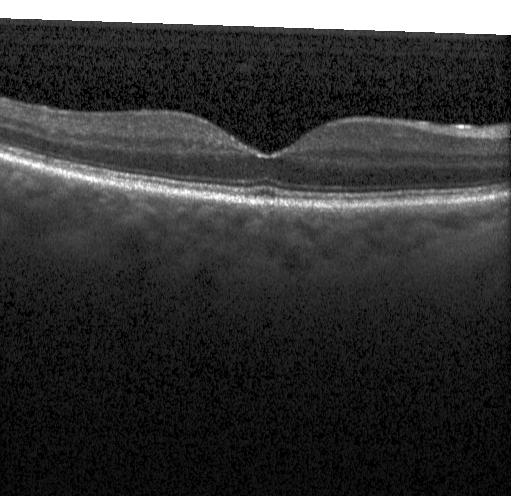 Through the macula, acquired on a Heidelberg Spectralis, OCT B-scan, spectral-domain optical coherence tomography. Diagnosis: no CNV, no DME, and no drusen.